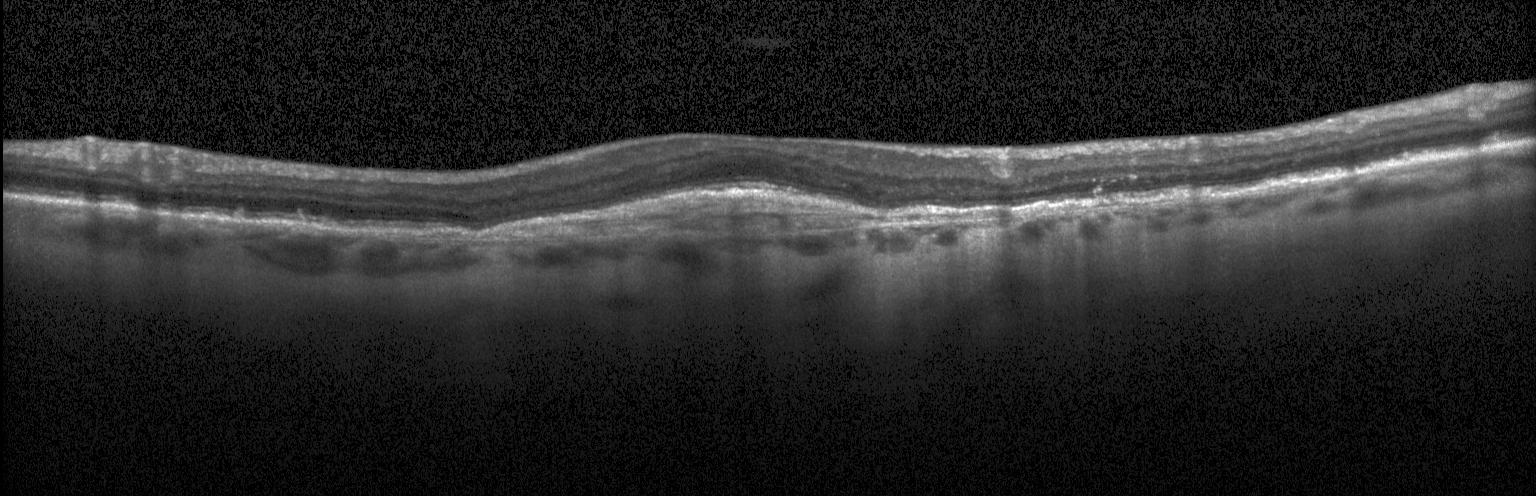 This B-scan demonstrates choroidal neovascularization.